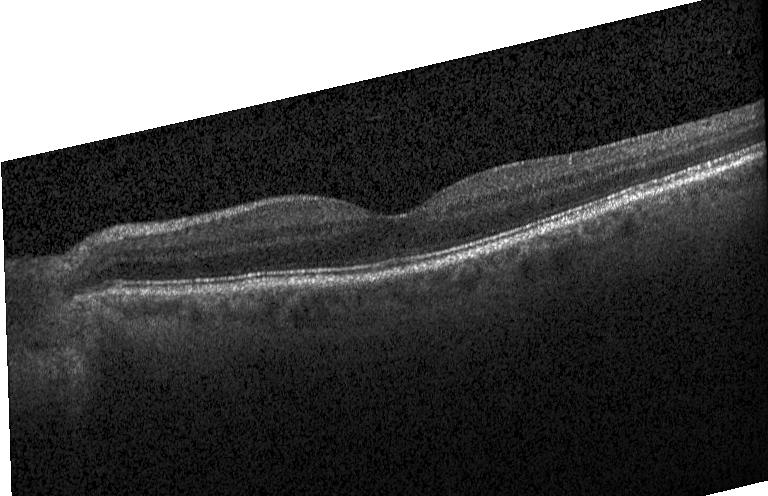
Heidelberg Spectralis, horizontal scan through the fovea, optical coherence tomography scan — The scan shows no choroidal neovascularization, diabetic macular edema, or drusen.